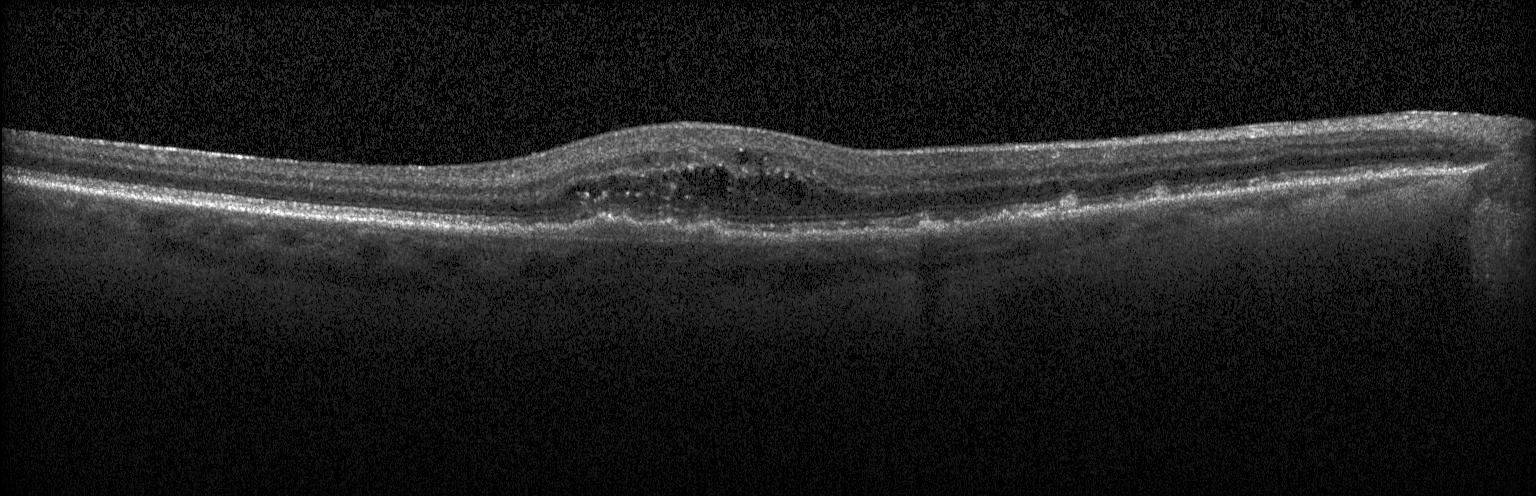 Retinal OCT B-scan. Finding: choroidal neovascularization (CNV).